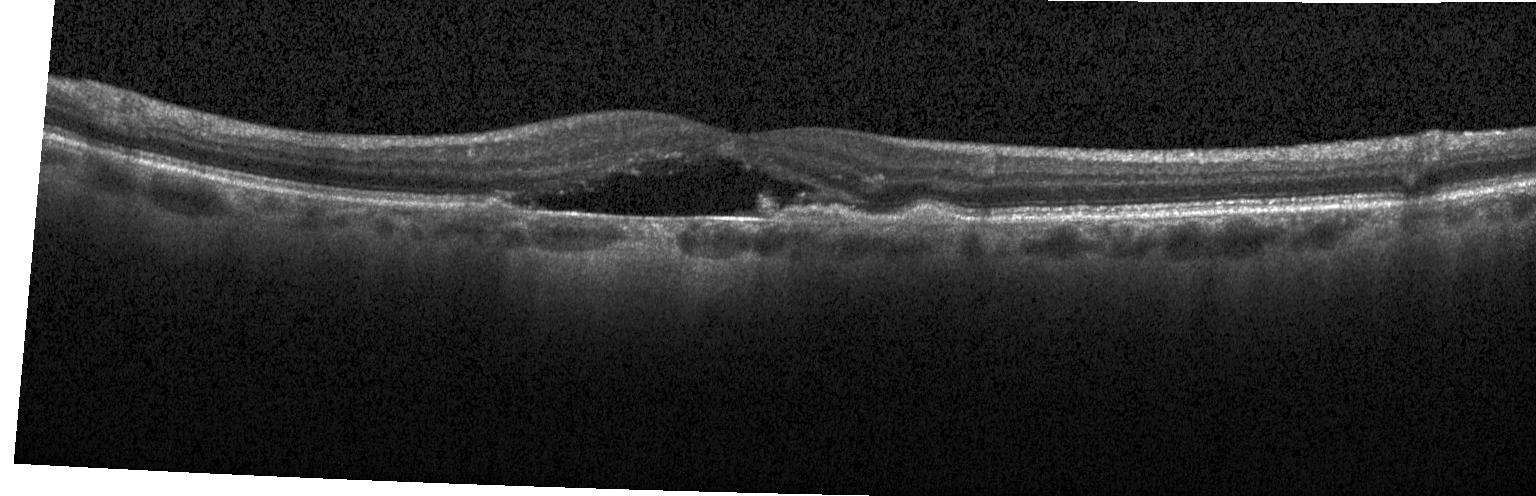 Spectral-domain OCT B-scan: choroidal neovascularization.